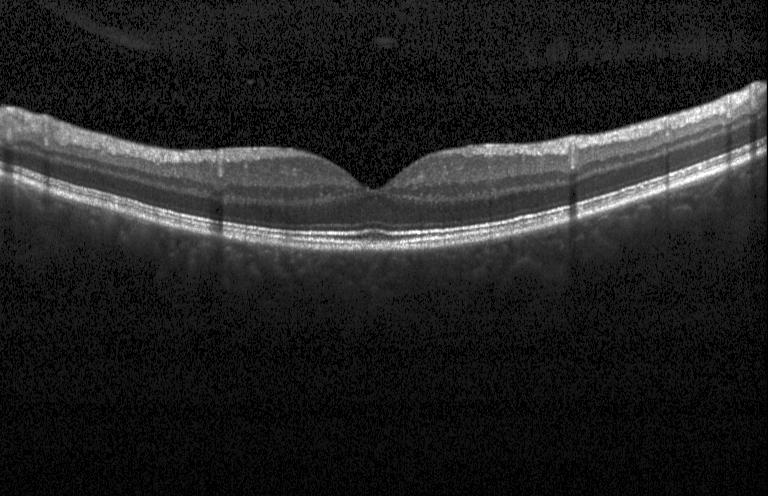 Macular OCT: no choroidal neovascularization, no diabetic macular edema, and no drusen.